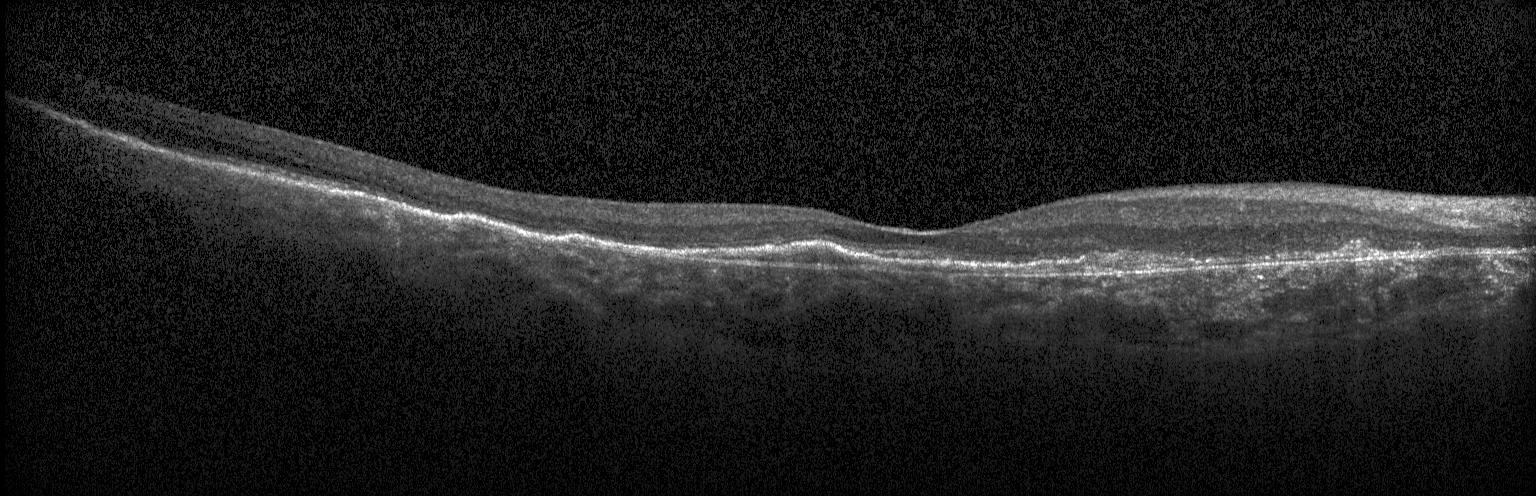 Macular OCT: a choroidal neovascular membrane.